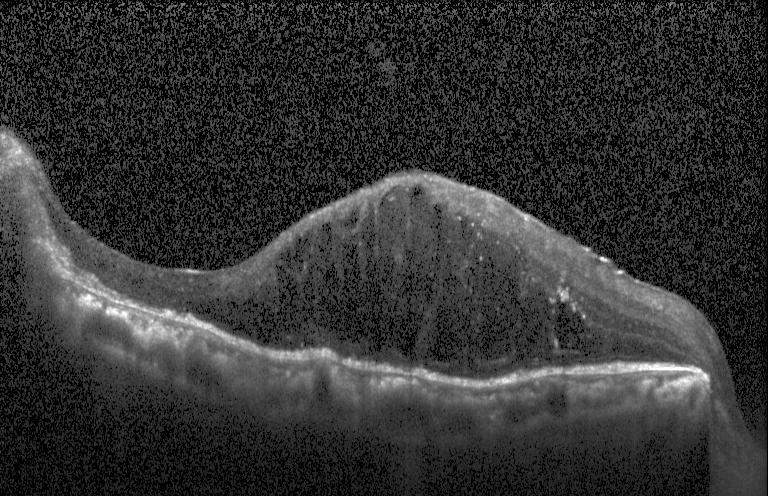
Optical coherence tomography scan; fovea-centered
Impression: DME.